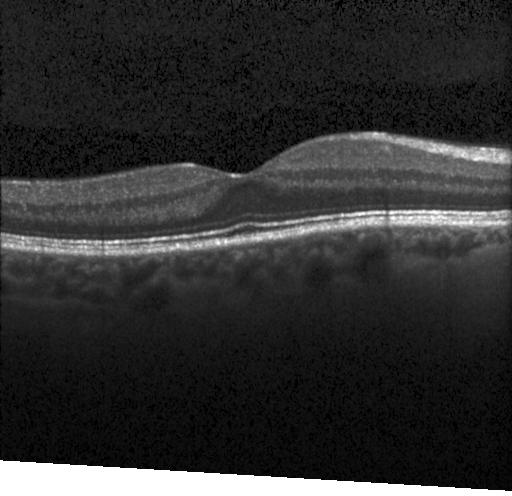
Macular scan · OCT line scan — Diagnosis: neither CNV, DME, nor drusen.